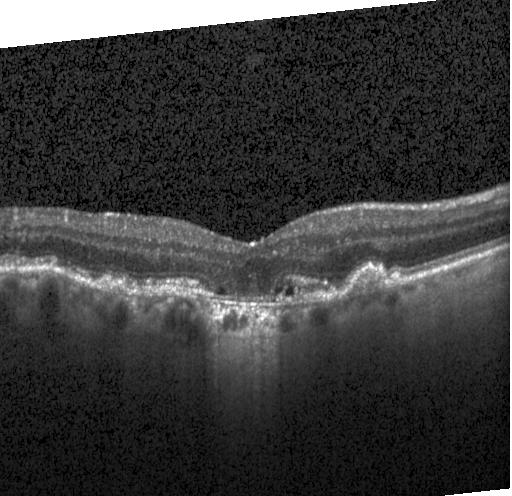

Centered on the fovea · Heidelberg Spectralis · OCT line scan — Diagnosis: a choroidal neovascular membrane.